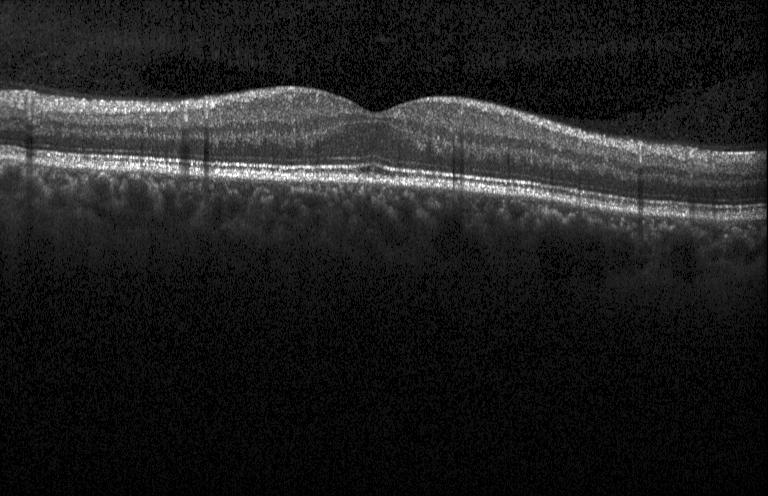

Macular OCT: neither choroidal neovascularization, diabetic macular edema, nor drusen.